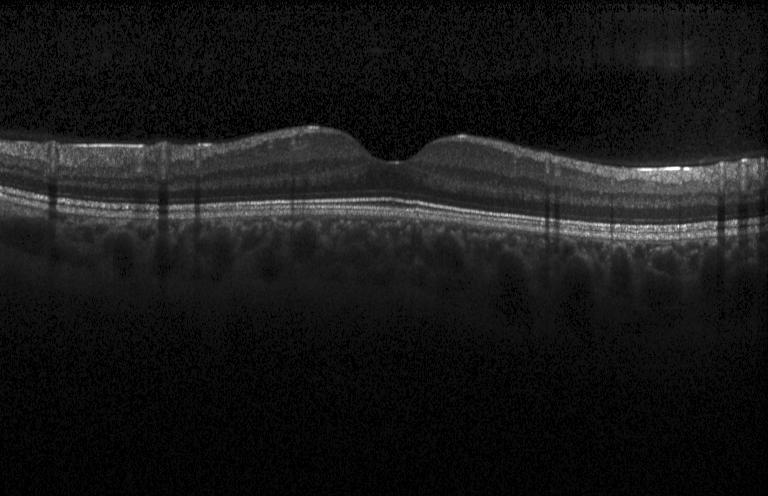

Spectral-domain optical coherence tomography · retinal OCT B-scan · Heidelberg Spectralis
This B-scan demonstrates no choroidal neovascularization, no diabetic macular edema, and no drusen.